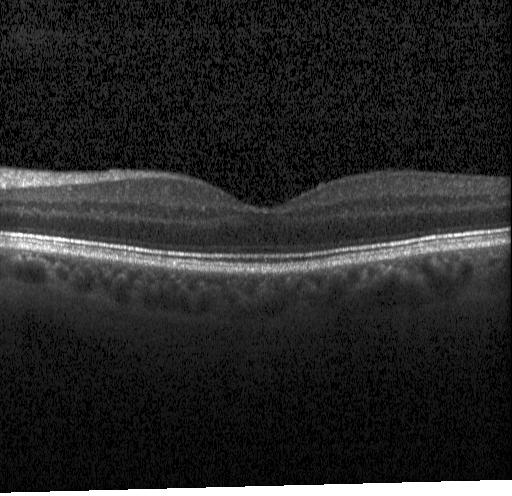
OCT B-scan showing neither choroidal neovascularization, diabetic macular edema, nor drusen.